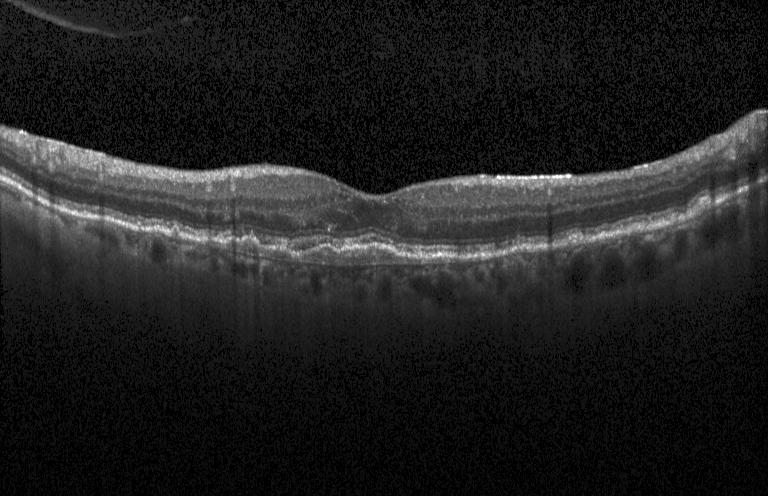
Optical coherence tomography scan — This B-scan demonstrates a choroidal neovascular membrane.